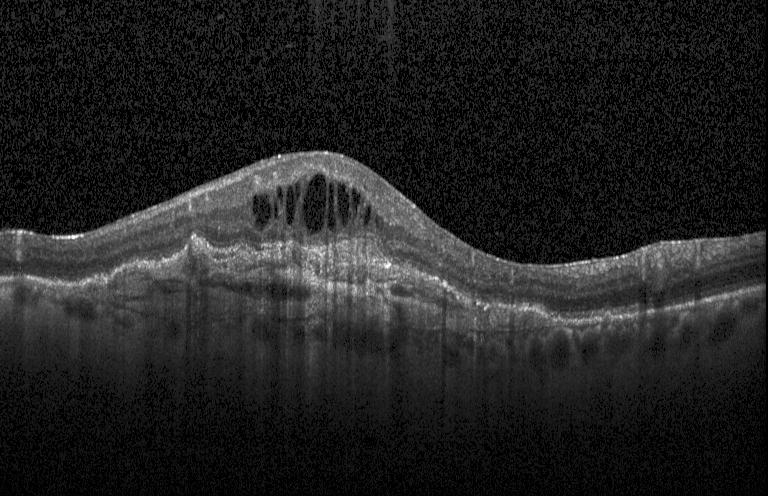 Spectral-domain OCT B-scan: a choroidal neovascular membrane.